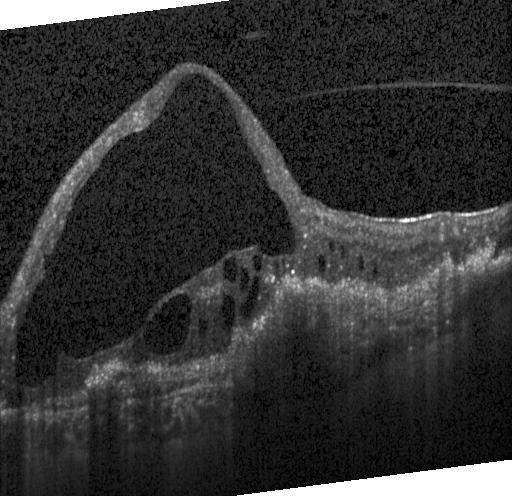
Retinal OCT B-scan, Heidelberg Spectralis OCT system
Macular OCT: a choroidal neovascular membrane.